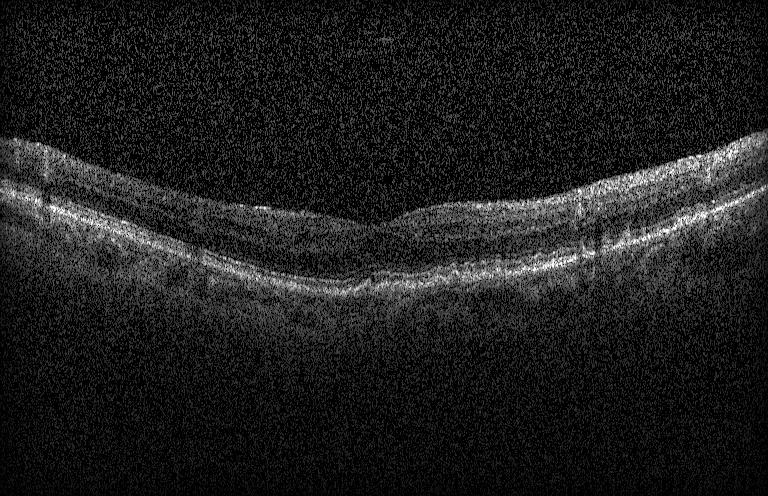 Dx: sub-RPE drusenoid deposits.